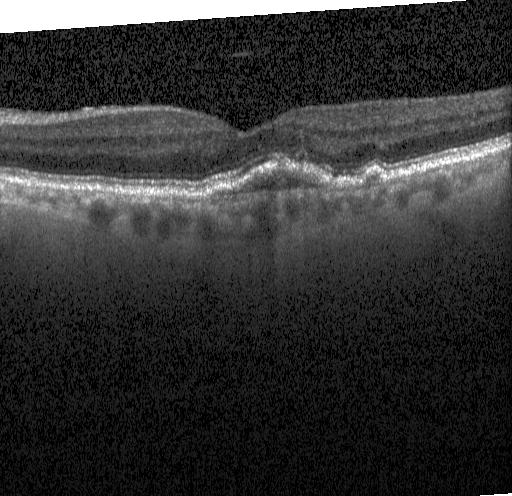 Retinal OCT B-scan — Finding: a choroidal neovascular membrane.